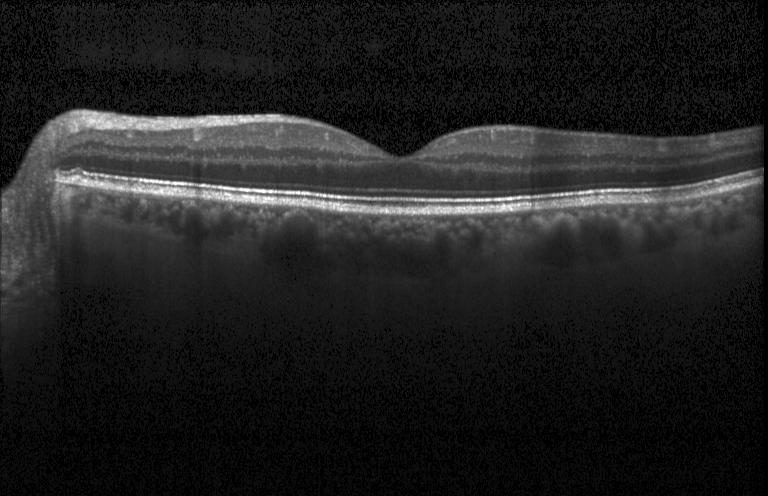

Fovea-centered. Spectral-domain optical coherence tomography. Optical coherence tomography B-scan — Diagnosis: neither CNV, DME, nor drusen.